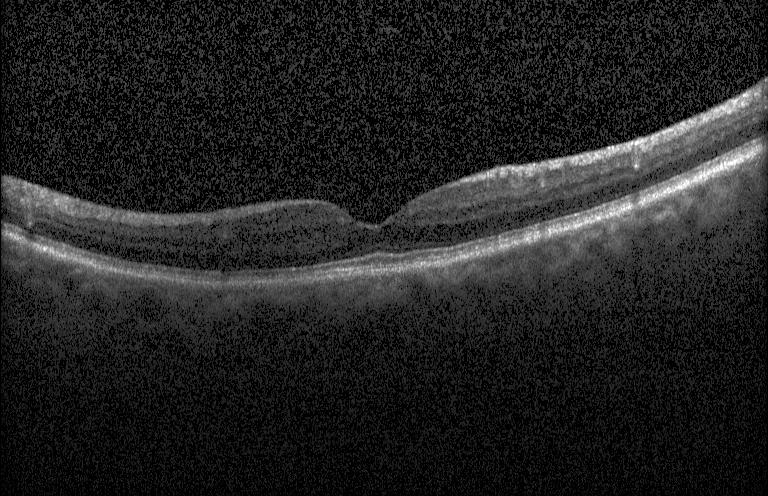

Optical coherence tomography B-scan
Impression: no choroidal neovascularization, diabetic macular edema, or drusen.